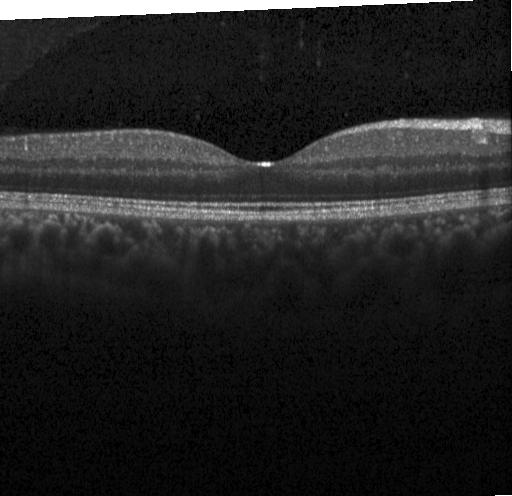
Impression: no evidence of choroidal neovascularization, diabetic macular edema, or drusen.